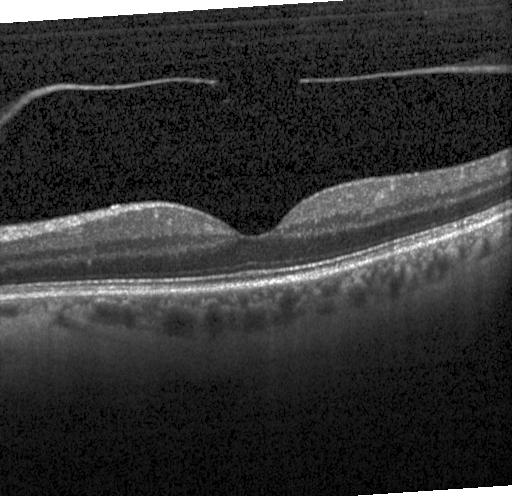 Retinal OCT cross-section. Impression: no CNV, DME, or drusen.